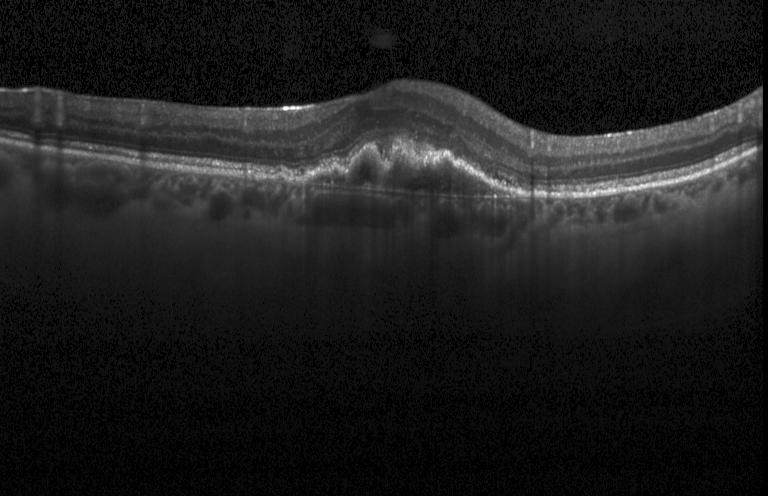 Spectral-domain OCT. Heidelberg Spectralis OCT system. OCT line scan. Macular scan. Dx: choroidal neovascularization (CNV).